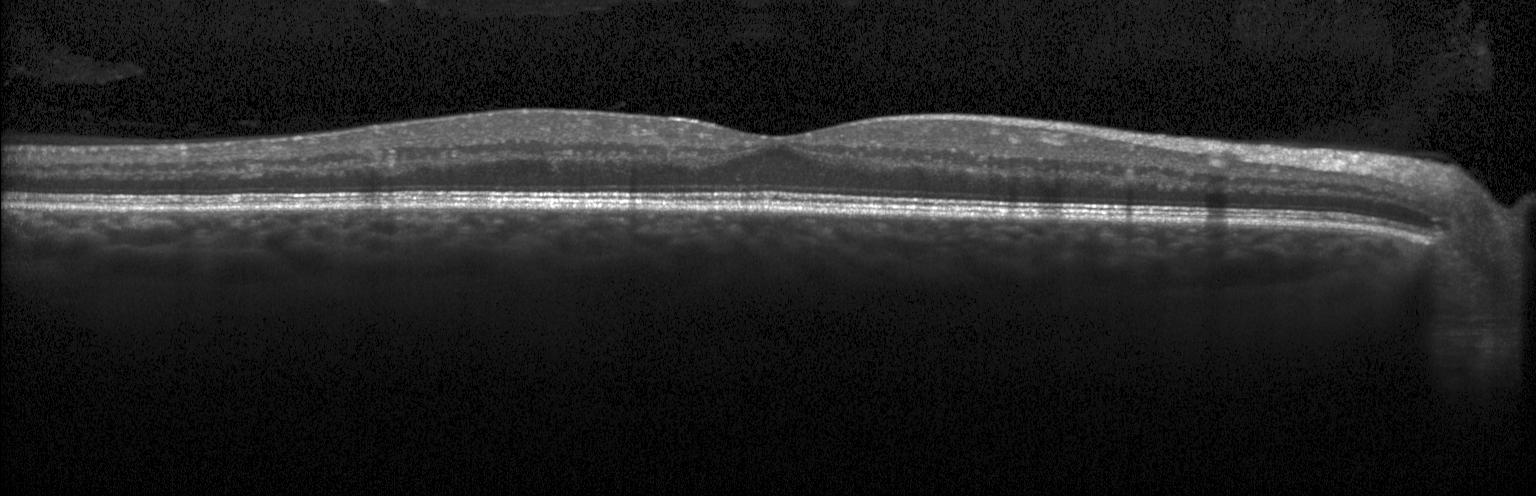

This B-scan demonstrates no evidence of CNV, DME, or drusen.